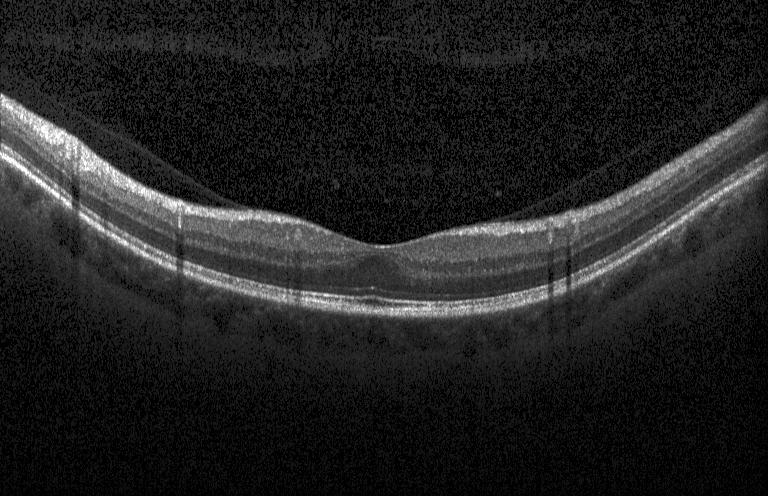
Macular OCT: no CNV, DME, or drusen.